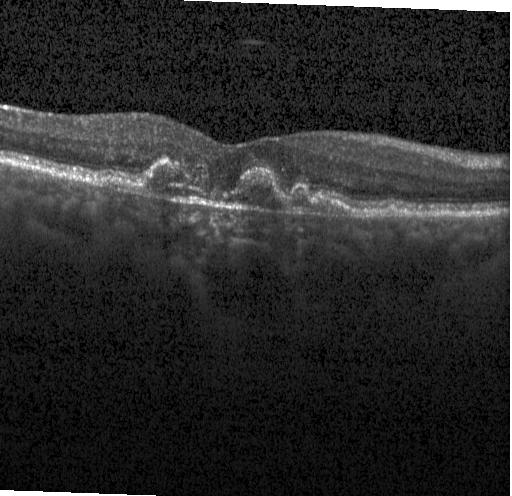

Impression: a choroidal neovascular membrane.